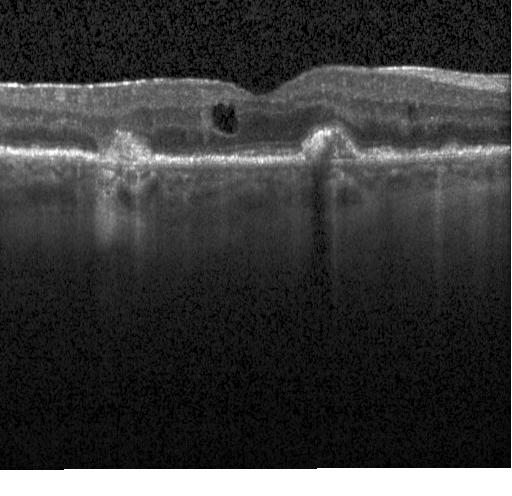
OCT B-scan — Impression: a choroidal neovascular membrane.